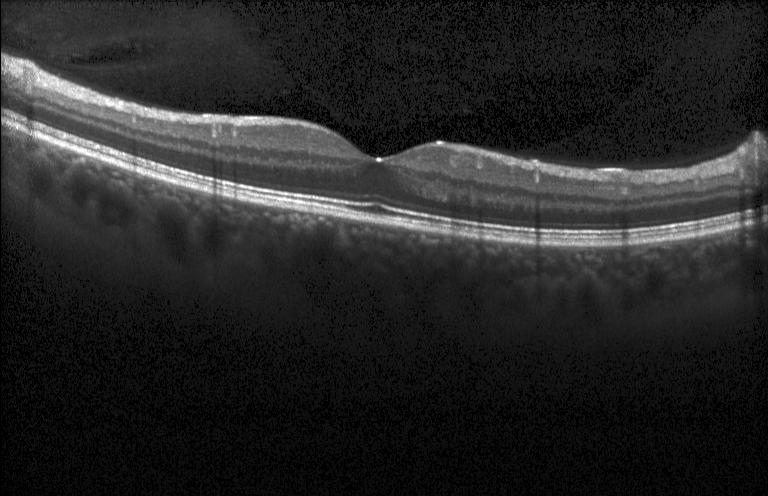

Retinal OCT cross-section
Dx: no evidence of choroidal neovascularization, diabetic macular edema, or drusen.